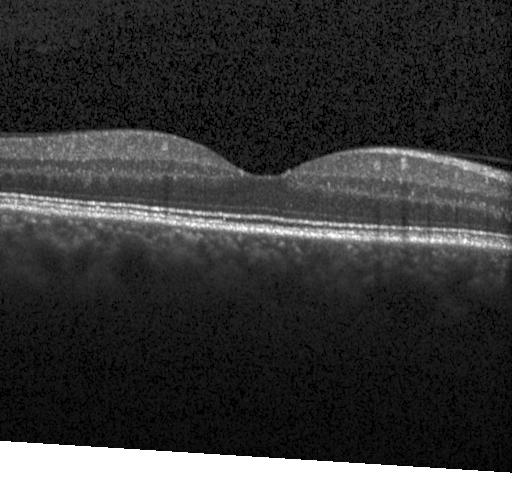
Optical coherence tomography B-scan. Heidelberg Spectralis OCT system. Macular OCT: no choroidal neovascularization, no diabetic macular edema, and no drusen.